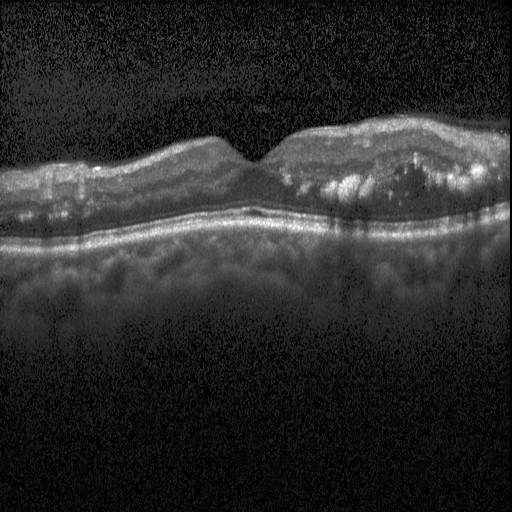
Optical coherence tomography scan, spectral-domain optical coherence tomography.
Dx: DME.